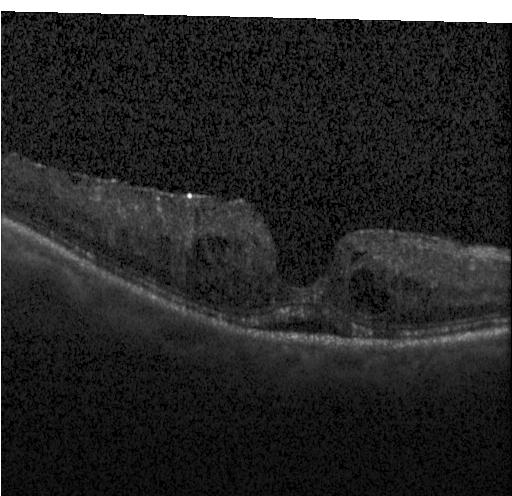
OCT finding: diabetic macular edema (DME).